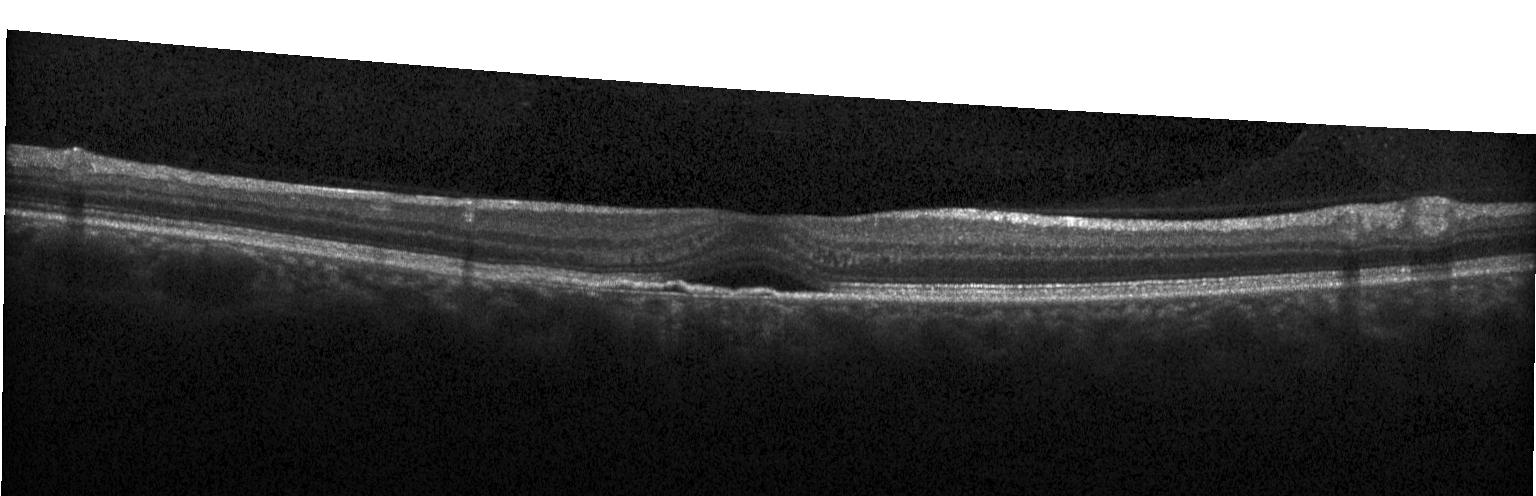

Spectral-domain OCT; OCT B-scan; instrument: Heidelberg Spectralis. Finding: choroidal neovascularization.